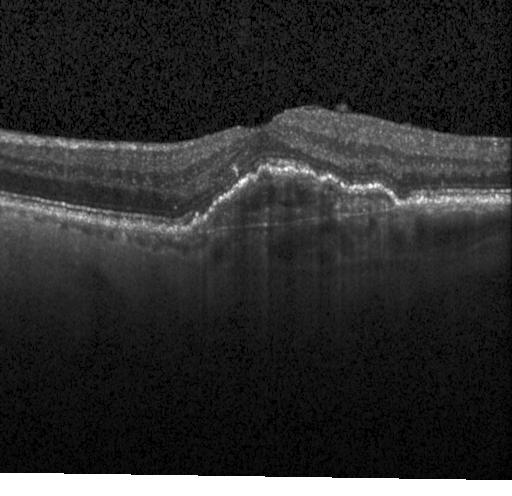 Spectral-domain optical coherence tomography, OCT B-scan, acquired on a Heidelberg Spectralis
A choroidal neovascular membrane.